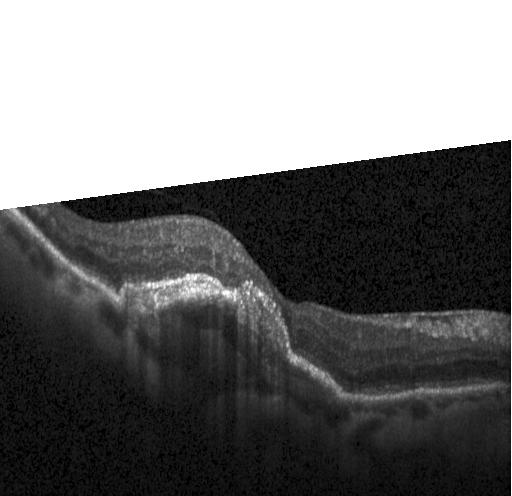
Spectral-domain OCT B-scan: CNV.